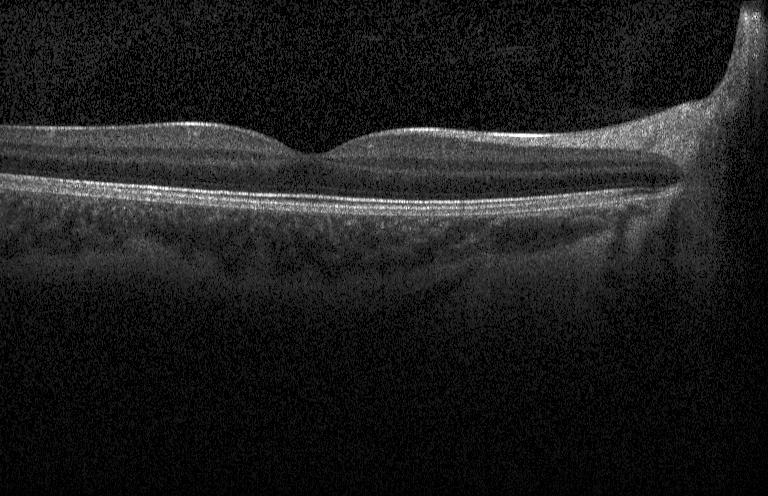

Macular scan, Heidelberg Spectralis OCT system, OCT B-scan, spectral-domain optical coherence tomography. Impression: no choroidal neovascularization, no diabetic macular edema, and no drusen.